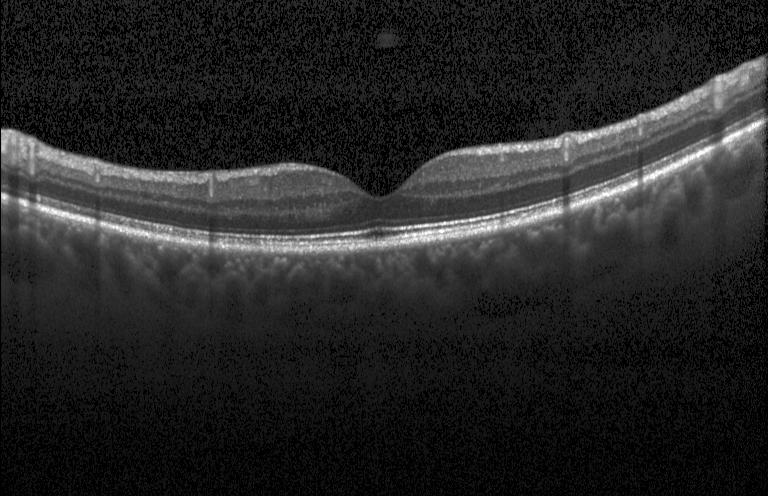

OCT B-scan showing no evidence of choroidal neovascularization, diabetic macular edema, or drusen.